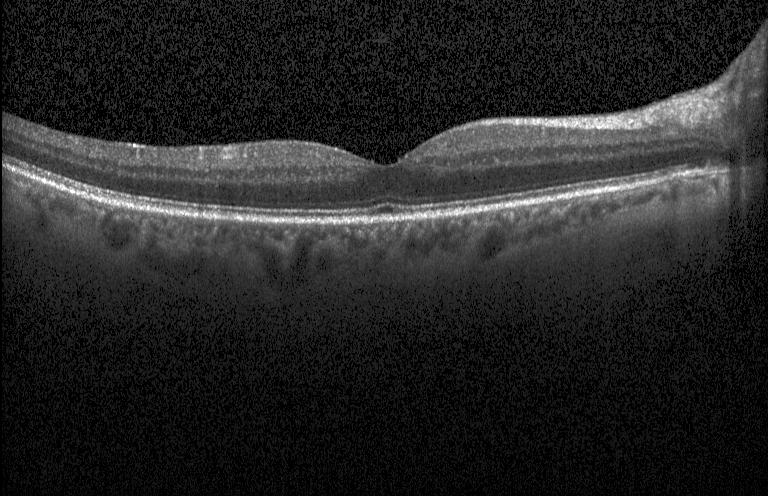 OCT line scan.
No CNV, DME, or drusen.